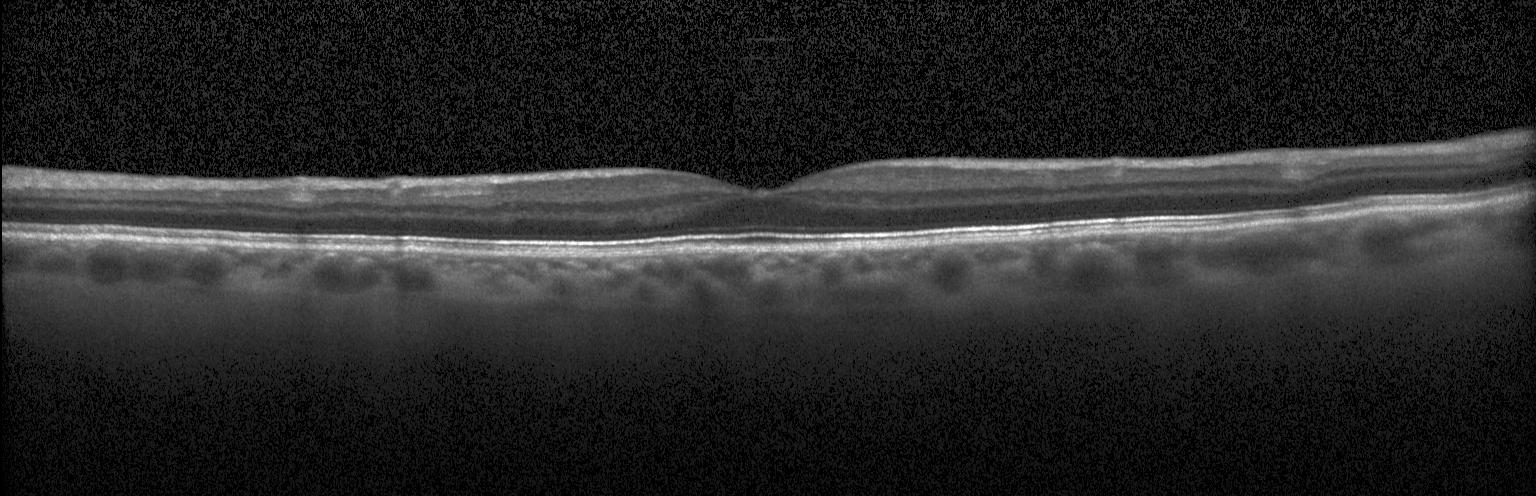 Instrument: Heidelberg Spectralis · OCT B-scan · horizontal scan through the fovea.
Diagnosis: no choroidal neovascularization, no diabetic macular edema, and no drusen.